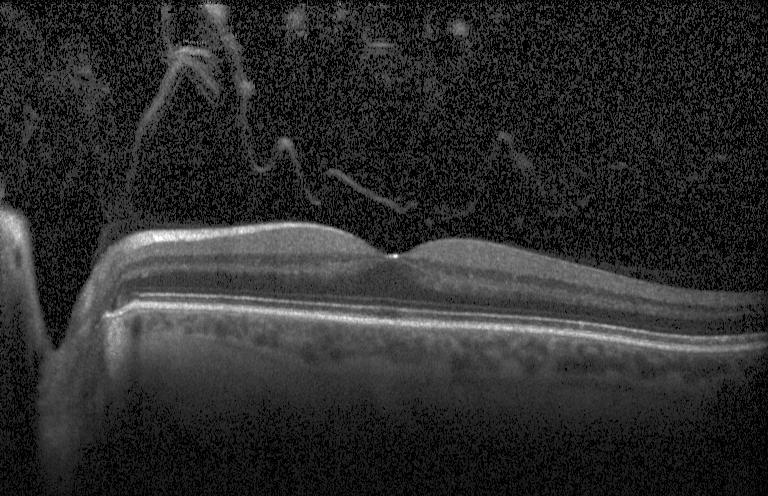
Assessment: neither CNV, DME, nor drusen.